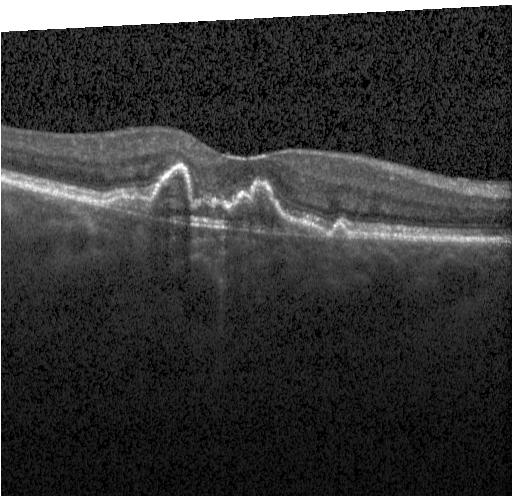
Centered on the fovea; optical coherence tomography B-scan. Impression: CNV.